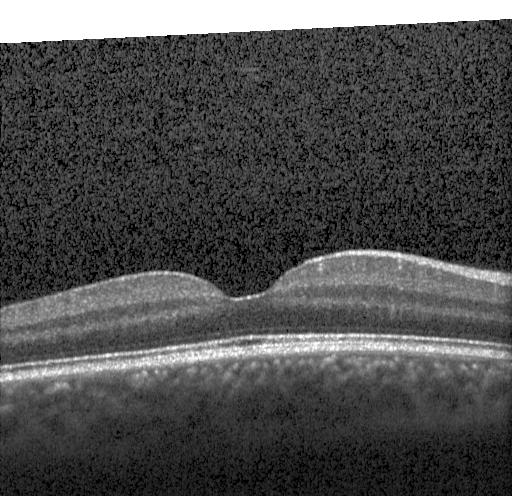 OCT B-scan.
This B-scan demonstrates neither choroidal neovascularization, diabetic macular edema, nor drusen.